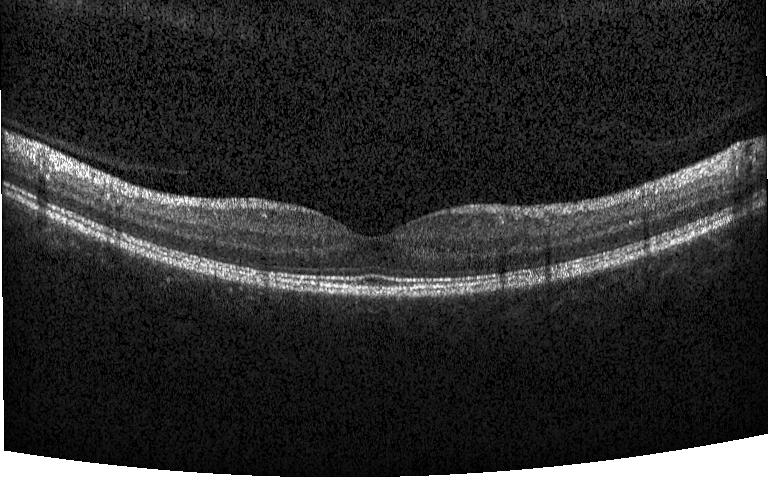

Retinal OCT B-scan — Macular OCT: neither CNV, DME, nor drusen.